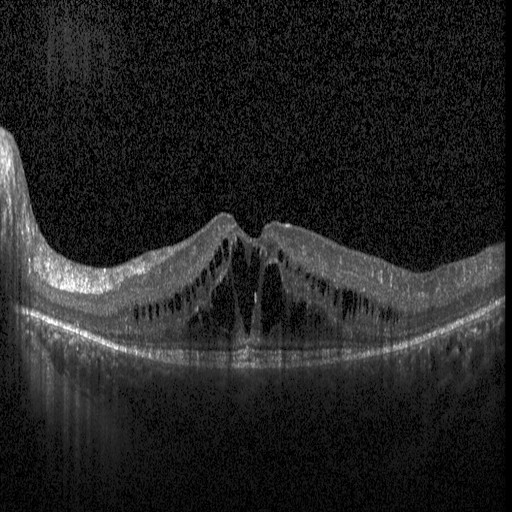
Spectral-domain optical coherence tomography, retinal OCT cross-section, Heidelberg Spectralis, fovea-centered. DME.